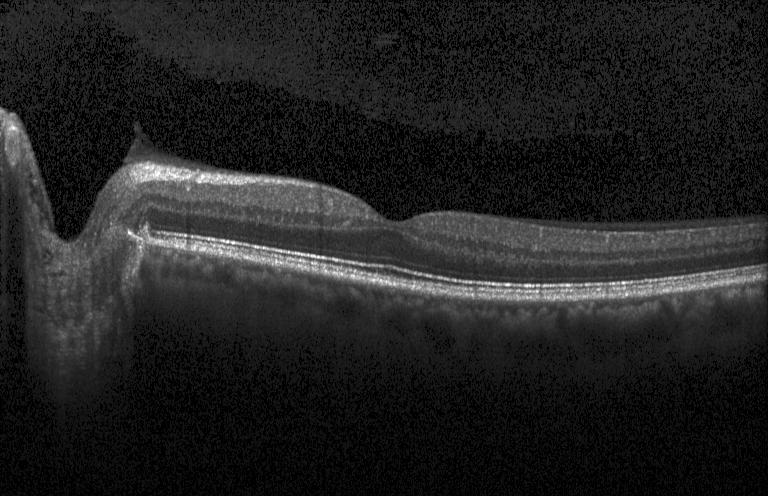
Optical coherence tomography scan — Impression: no evidence of choroidal neovascularization, diabetic macular edema, or drusen.